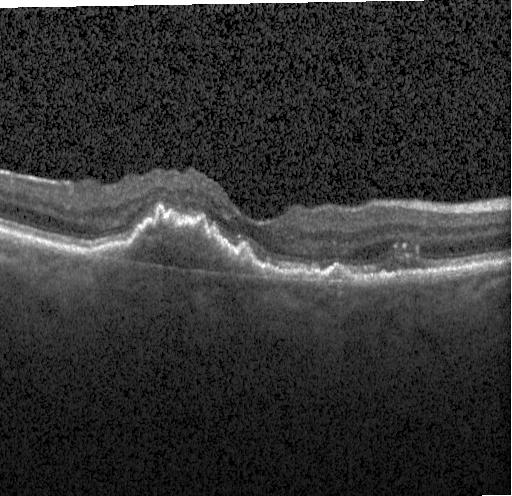
Macular OCT: a choroidal neovascular membrane.